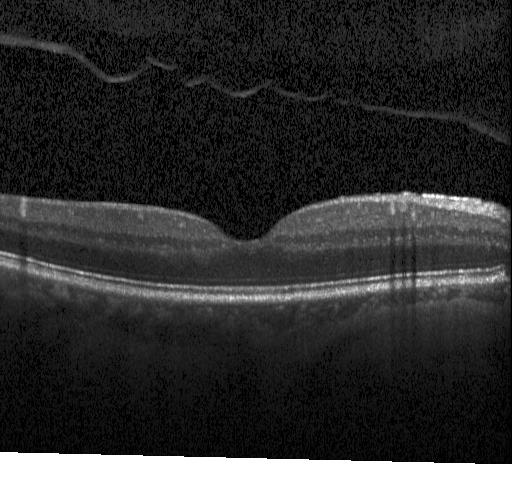 Heidelberg Spectralis OCT system. Optical coherence tomography scan.
Finding: no choroidal neovascularization, diabetic macular edema, or drusen.